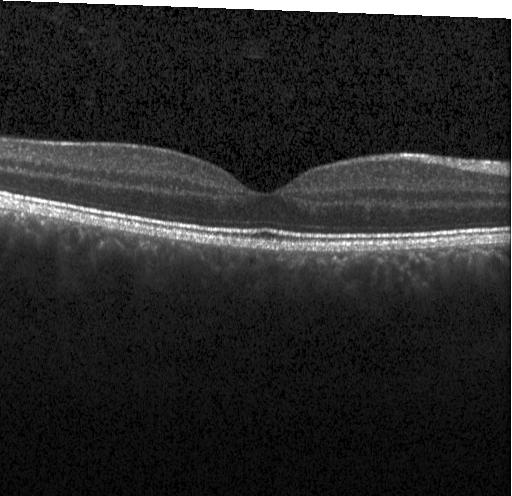 Assessment: no evidence of CNV, DME, or drusen.